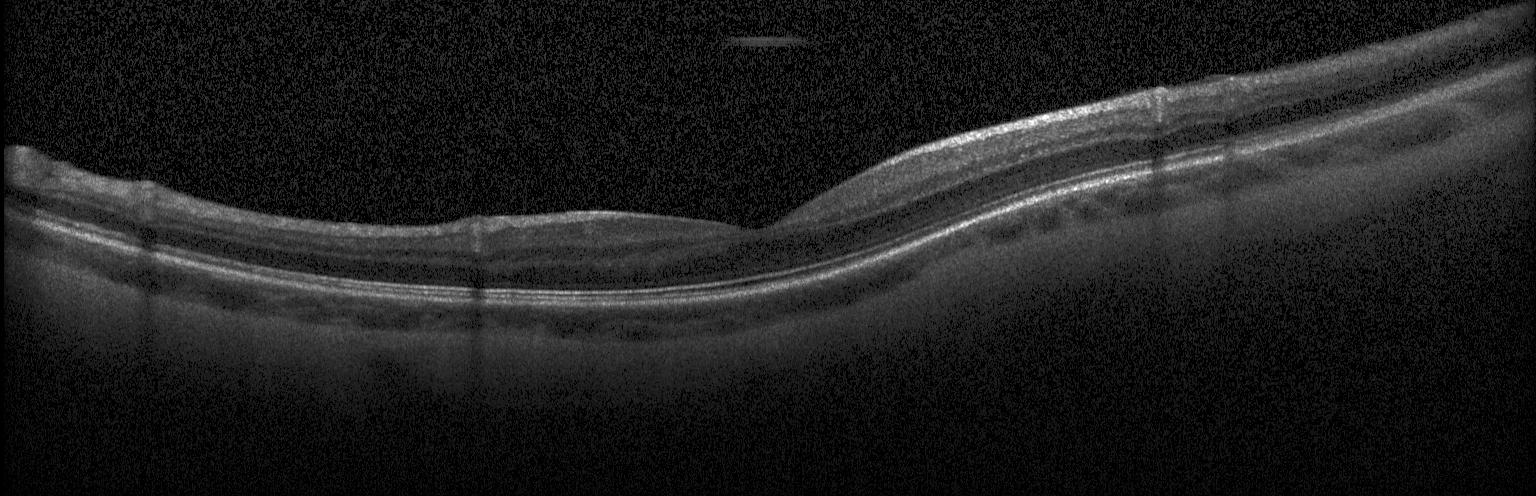
Neither CNV, DME, nor drusen.